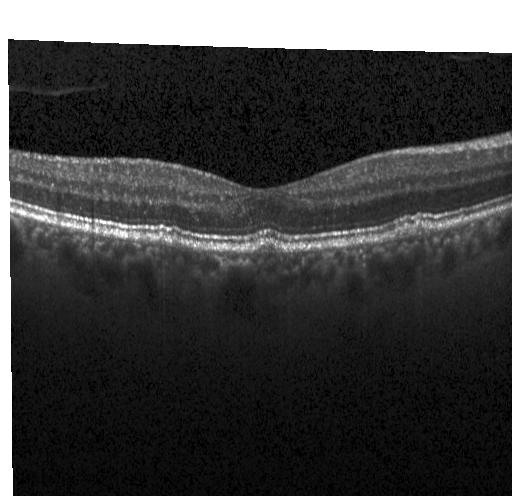 Retinal OCT cross-section showing drusen.